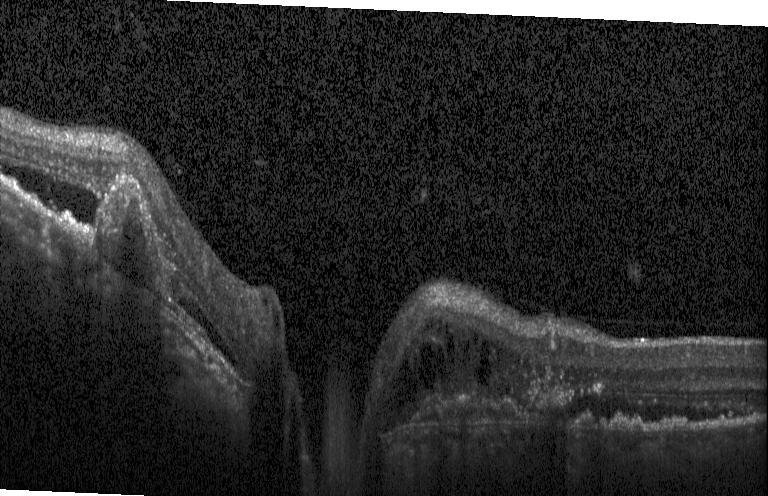
Optical coherence tomography scan · Heidelberg Spectralis OCT system · SD-OCT. A choroidal neovascular membrane.